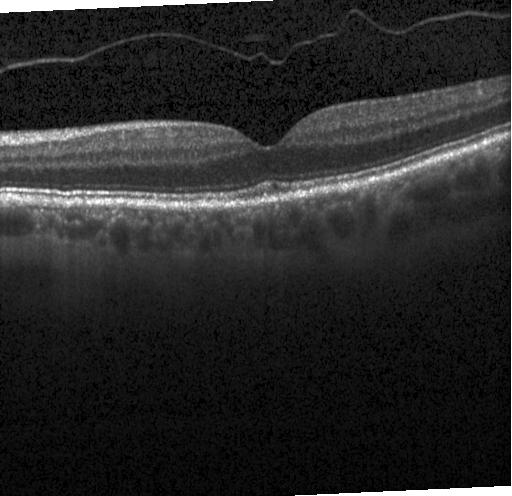

Retinal OCT B-scan; centered on the fovea — Diagnosis: no choroidal neovascularization, no diabetic macular edema, and no drusen.